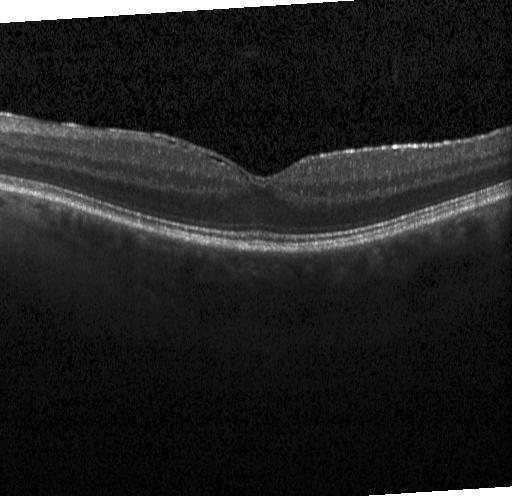
OCT line scan. Spectral-domain optical coherence tomography. Macular scan. Heidelberg Spectralis OCT system.
Diagnosis: neither CNV, DME, nor drusen.